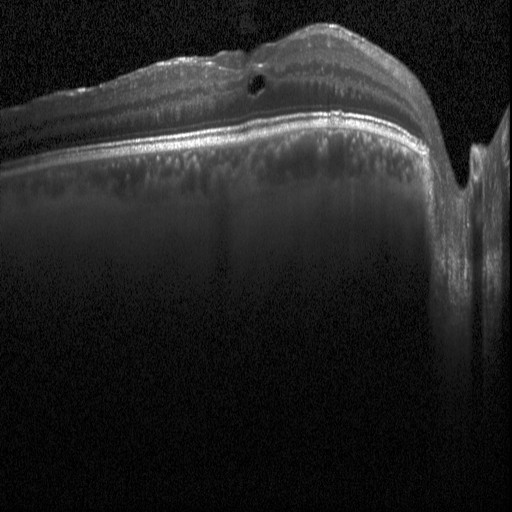 Heidelberg Spectralis OCT system; OCT line scan; macular scan
Impression: diabetic macular edema.